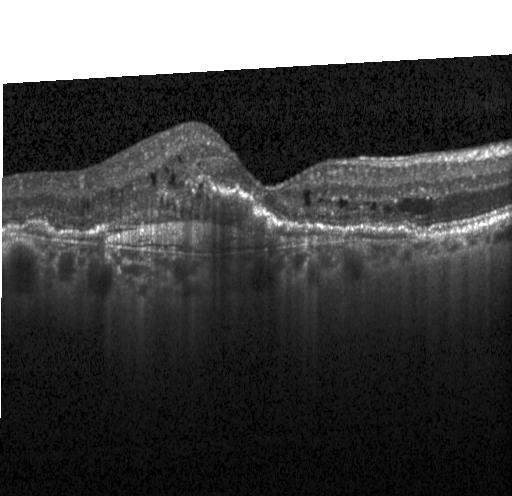 Heidelberg Spectralis. Optical coherence tomography B-scan. SD-OCT. Horizontal scan through the fovea.
Choroidal neovascularization.